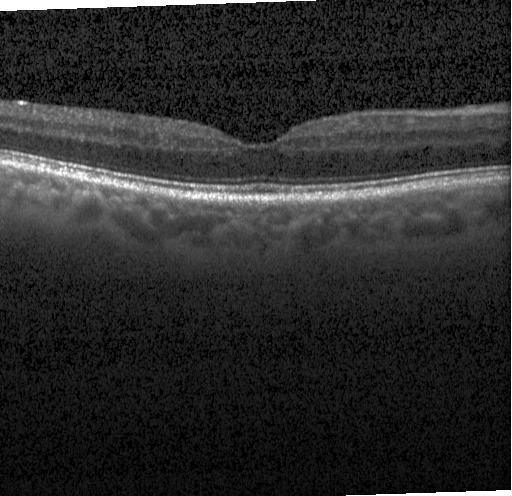

Acquired on a Heidelberg Spectralis, spectral-domain OCT, OCT line scan, horizontal scan through the fovea.
Impression: no CNV, DME, or drusen.